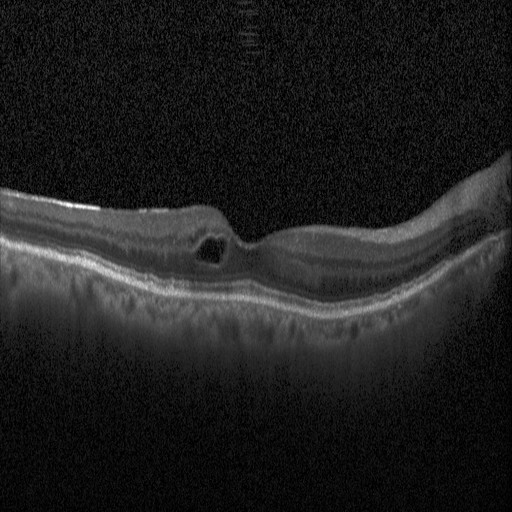 Macular OCT: diabetic macular edema.